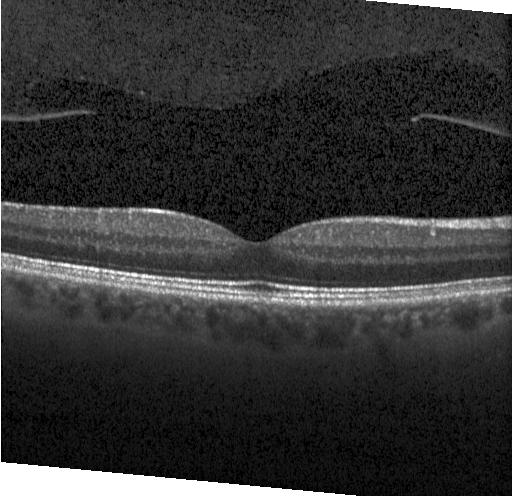 Retinal OCT cross-section. The scan shows neither choroidal neovascularization, diabetic macular edema, nor drusen.